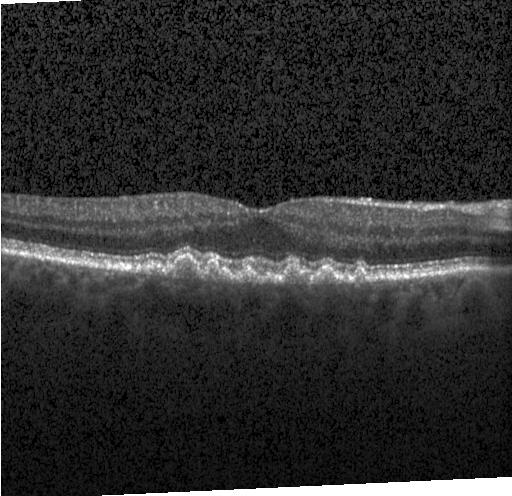 Impression: drusen.